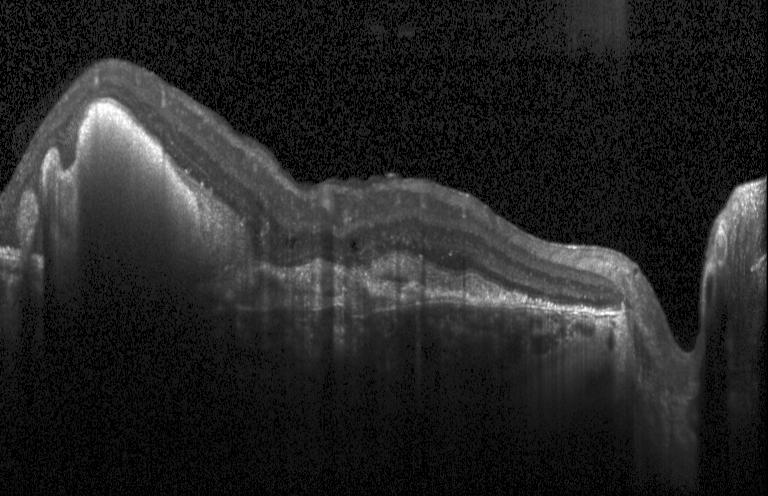 Optical coherence tomography B-scan; fovea-centered; spectral-domain OCT. Macular OCT: a choroidal neovascular membrane.